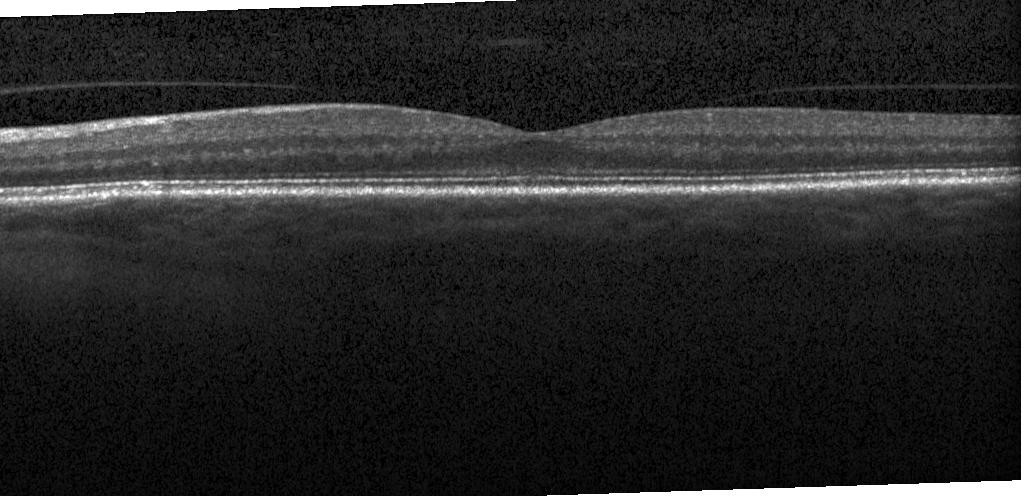 Horizontal scan through the fovea, OCT line scan, SD-OCT.
Impression: no CNV, DME, or drusen.